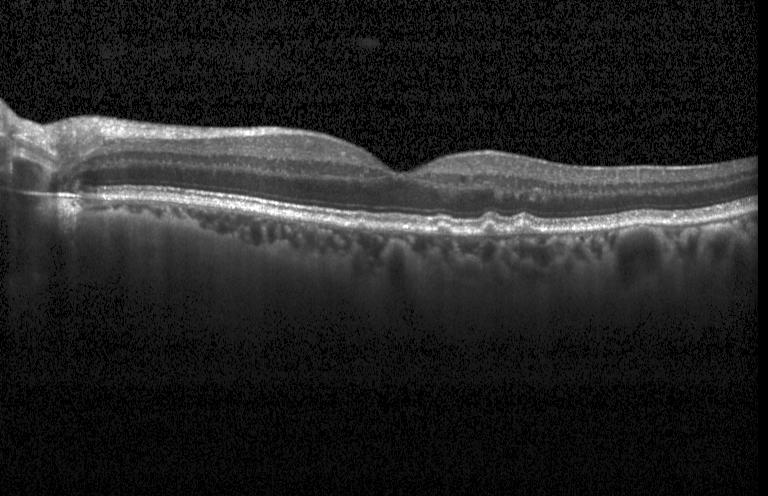

Retinal OCT B-scan. Macular scan. Spectral-domain OCT
Impression: multiple drusen.